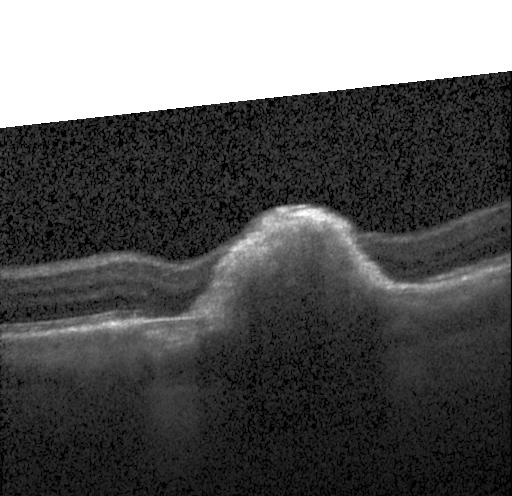
OCT line scan. Finding: choroidal neovascularization (CNV).